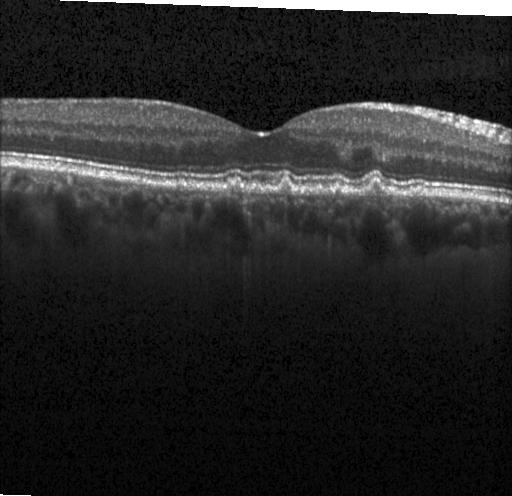

Spectral-domain optical coherence tomography, OCT B-scan, horizontal scan through the fovea. Dx: multiple drusen.